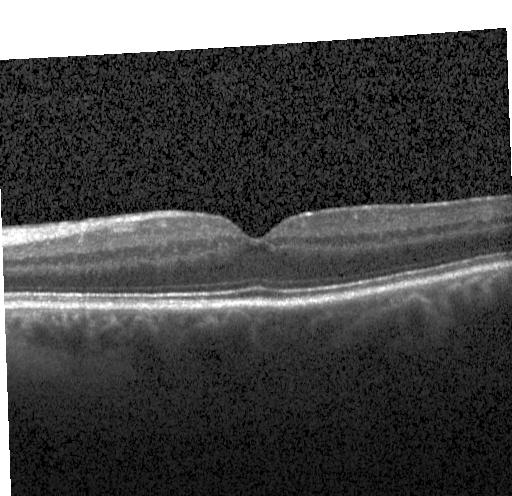

Heidelberg Spectralis OCT system; SD-OCT; OCT B-scan — Macular OCT: no evidence of choroidal neovascularization, diabetic macular edema, or drusen.